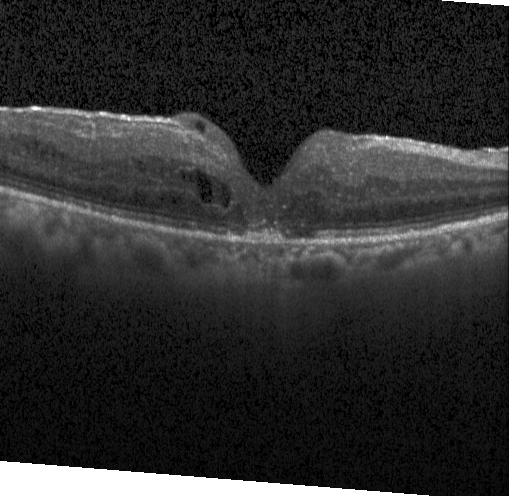
Macular OCT demonstrating diabetic macular edema.